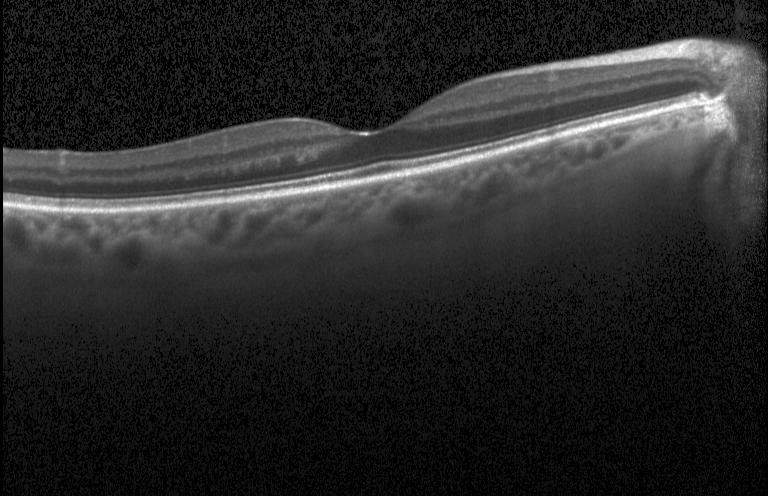
Impression: neither choroidal neovascularization, diabetic macular edema, nor drusen.